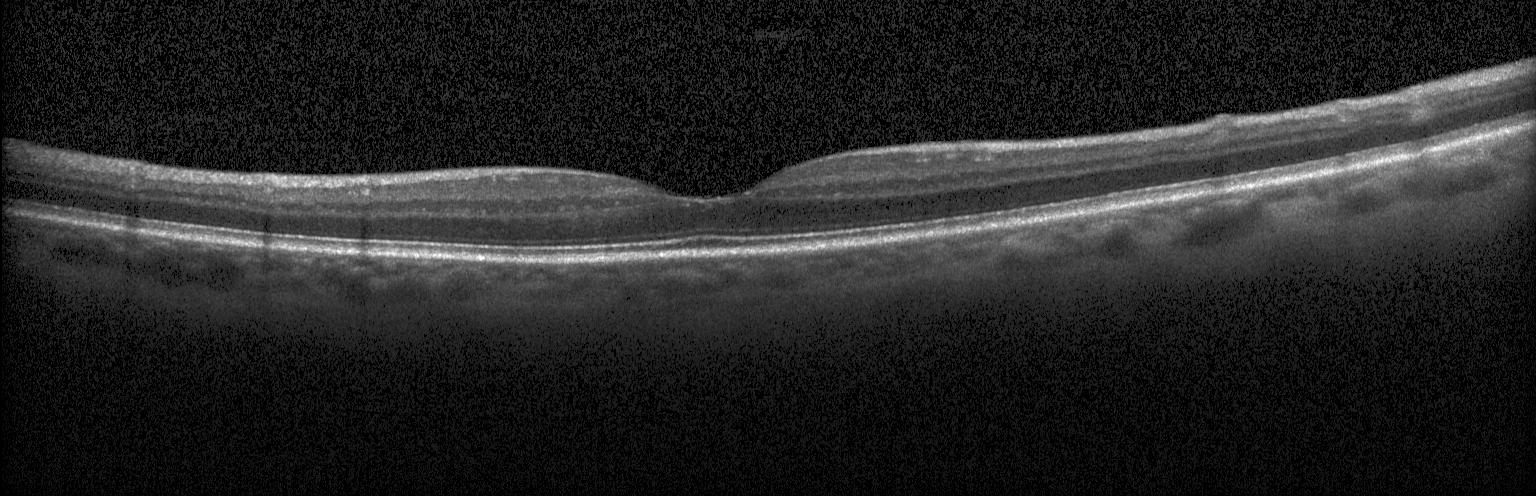

Acquired on a Heidelberg Spectralis · OCT line scan
Diagnosis: neither CNV, DME, nor drusen.